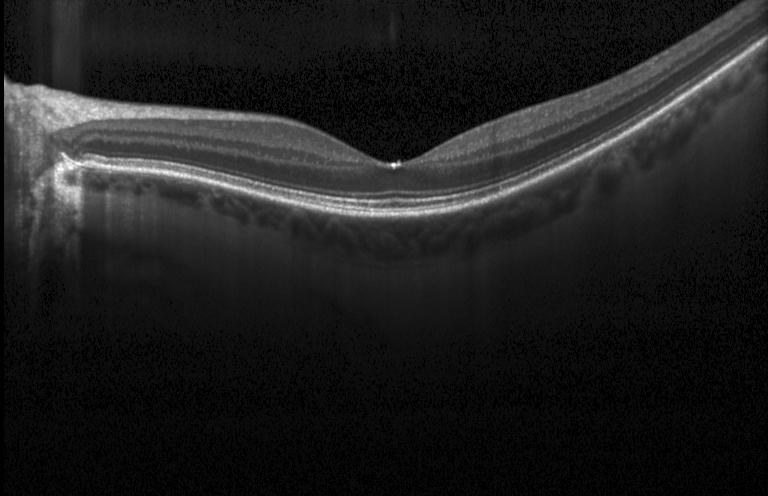
Retinal OCT B-scan
Diagnosis: no evidence of choroidal neovascularization, diabetic macular edema, or drusen.